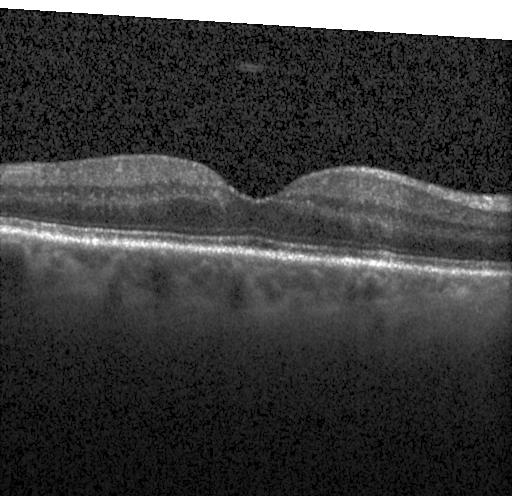

Optical coherence tomography B-scan, instrument: Heidelberg Spectralis — Dx: neither CNV, DME, nor drusen.